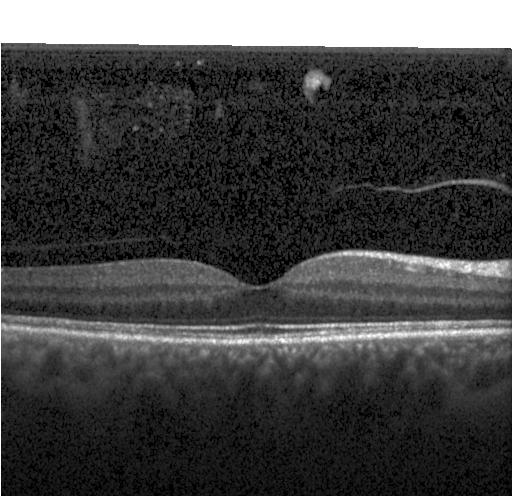 Optical coherence tomography scan — OCT finding: no choroidal neovascularization, diabetic macular edema, or drusen.